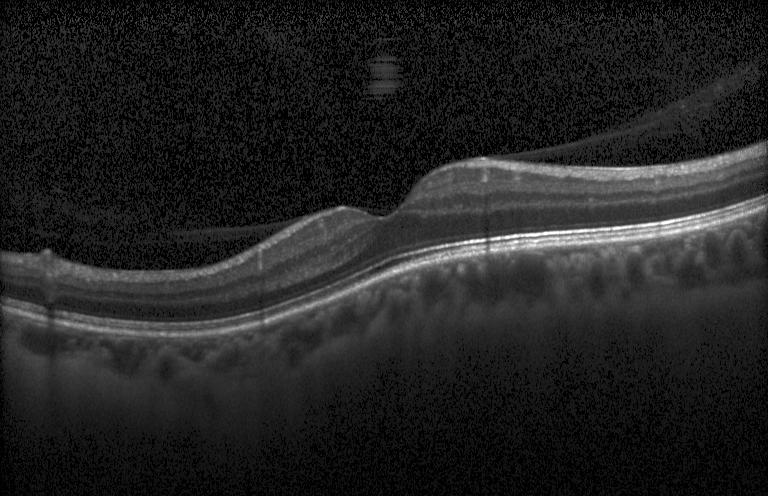 Optical coherence tomography B-scan.
No evidence of CNV, DME, or drusen.